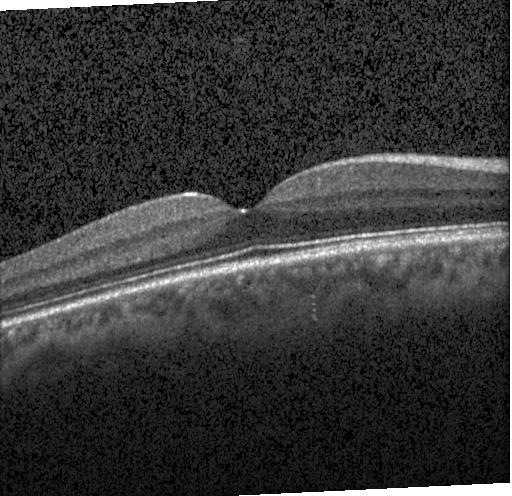 Assessment: no choroidal neovascularization, diabetic macular edema, or drusen.